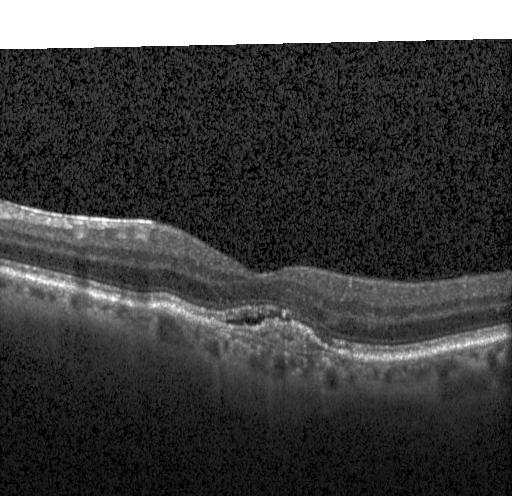

Retinal OCT cross-section
The scan shows a choroidal neovascular membrane.